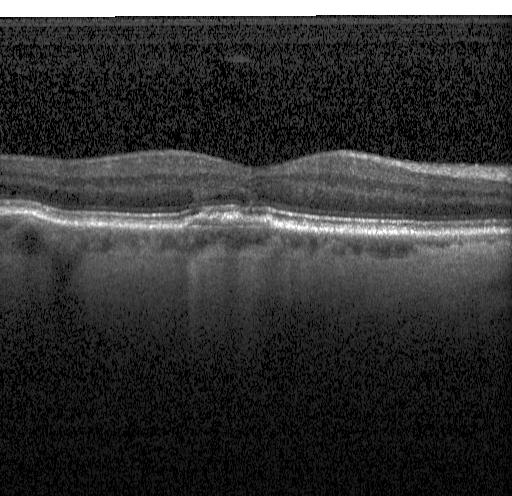
Diagnosis: a choroidal neovascular membrane.